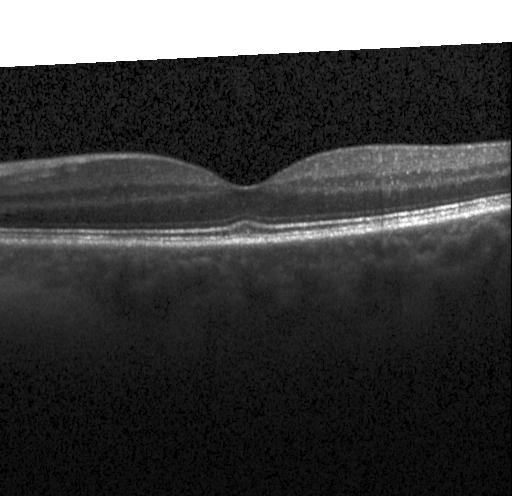

Spectral-domain OCT B-scan: no CNV, no DME, and no drusen.